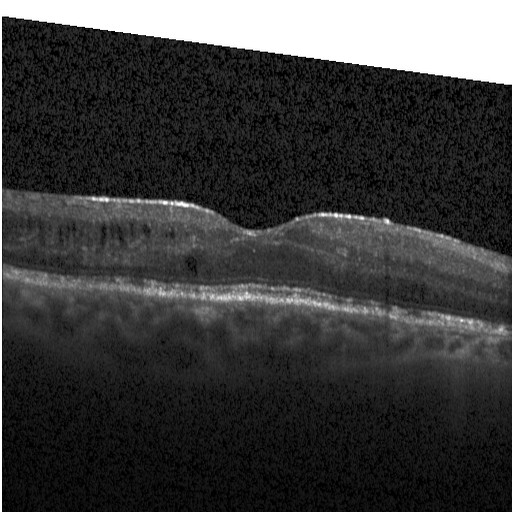 Diagnosis: DME.